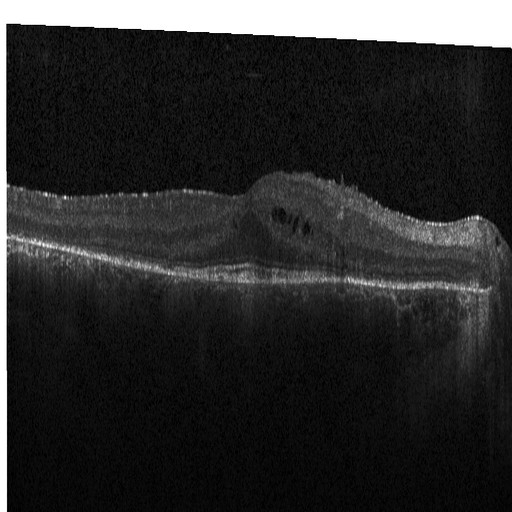 Macular OCT demonstrating diabetic macular edema.